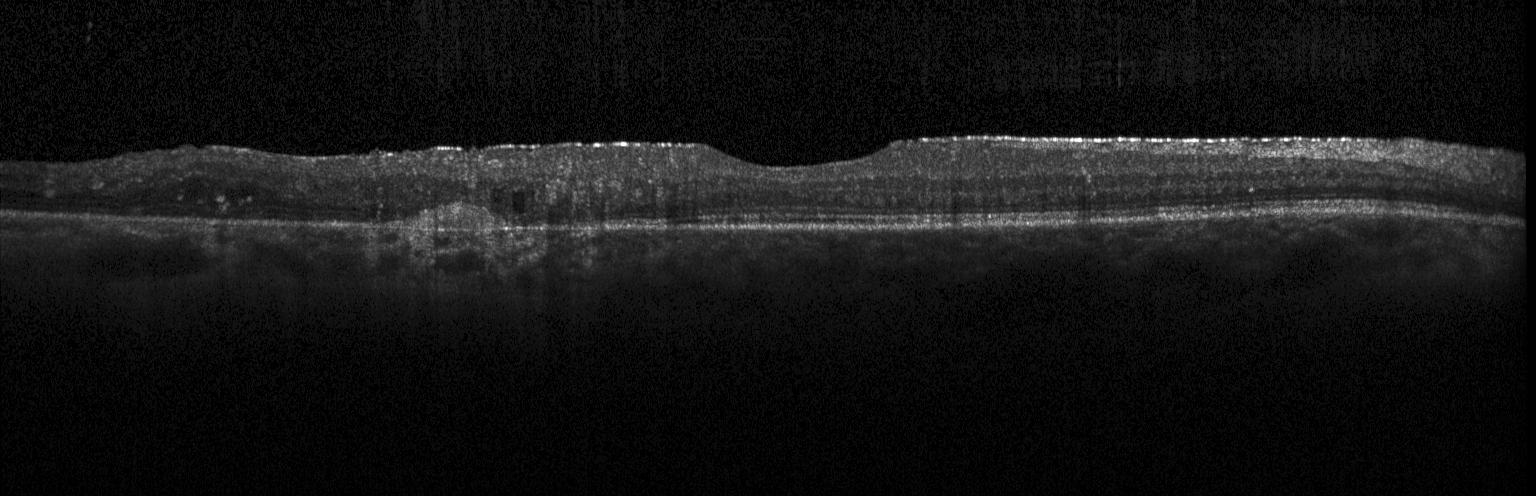 This B-scan demonstrates a choroidal neovascular membrane.